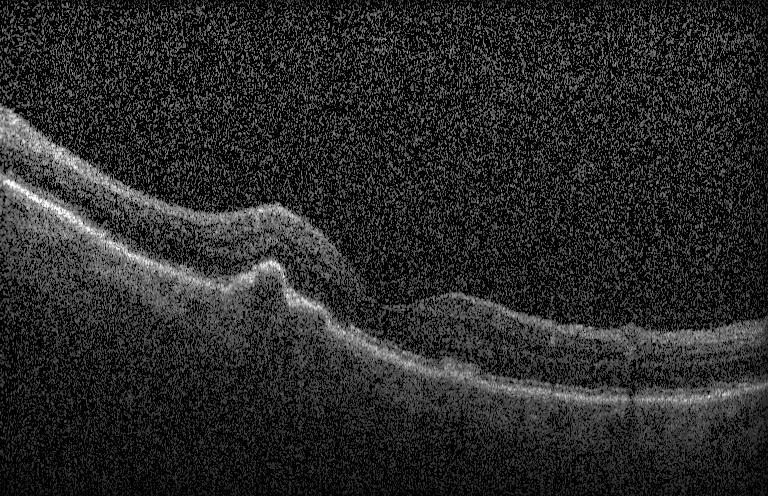

OCT scan showing a choroidal neovascular membrane.